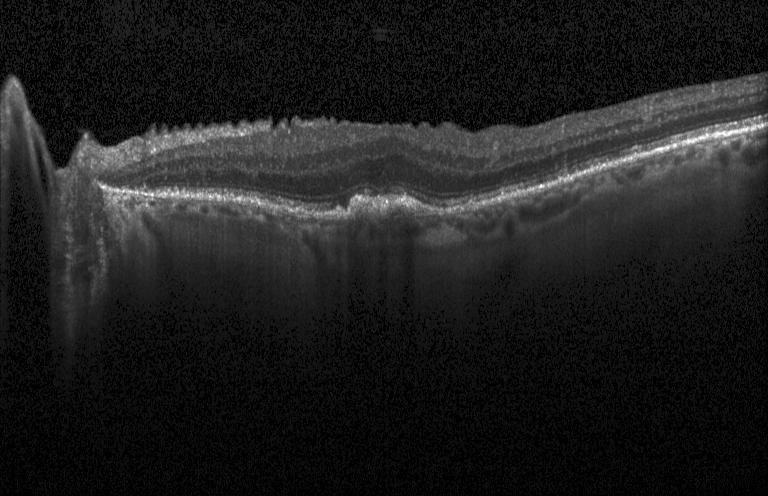

Centered on the fovea, optical coherence tomography B-scan.
Diagnosis: a choroidal neovascular membrane.